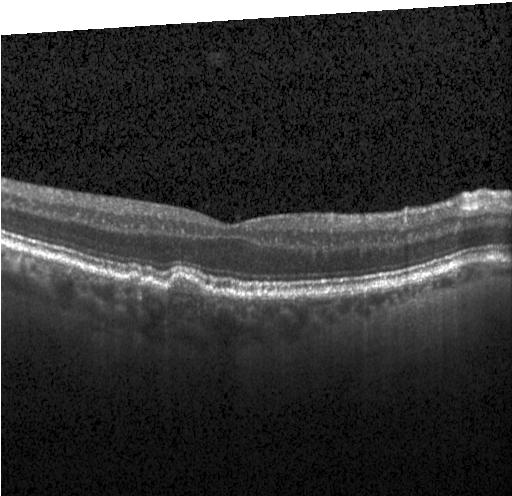
Horizontal scan through the fovea. Retinal OCT B-scan — Diagnosis: drusen.